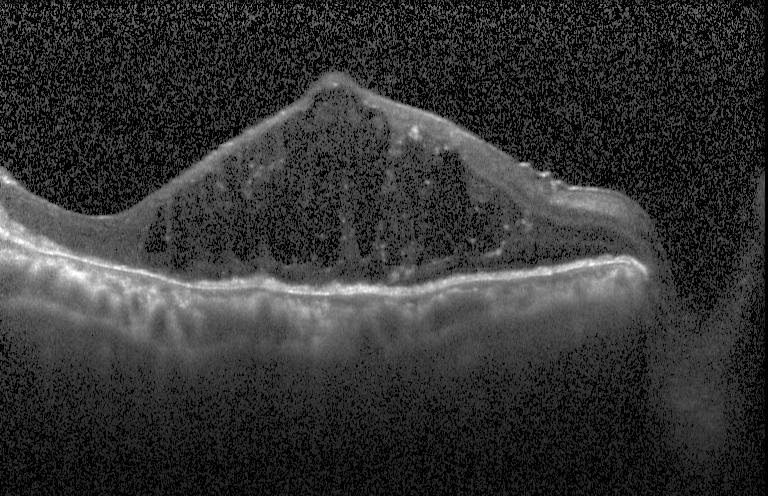

Retinal OCT B-scan, macular scan, spectral-domain optical coherence tomography, instrument: Heidelberg Spectralis — This B-scan demonstrates diabetic macular edema.